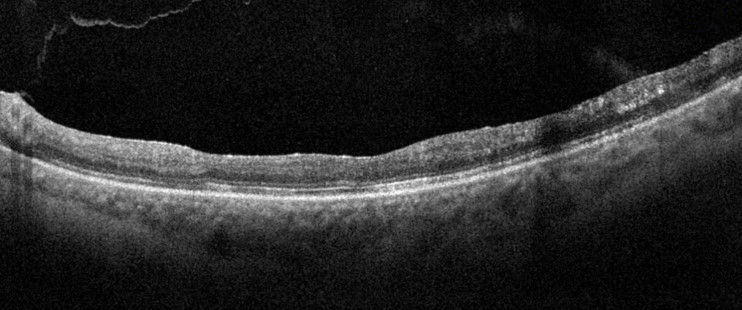
Retinal OCT cross-section. Finding: diabetic macular edema (DME).